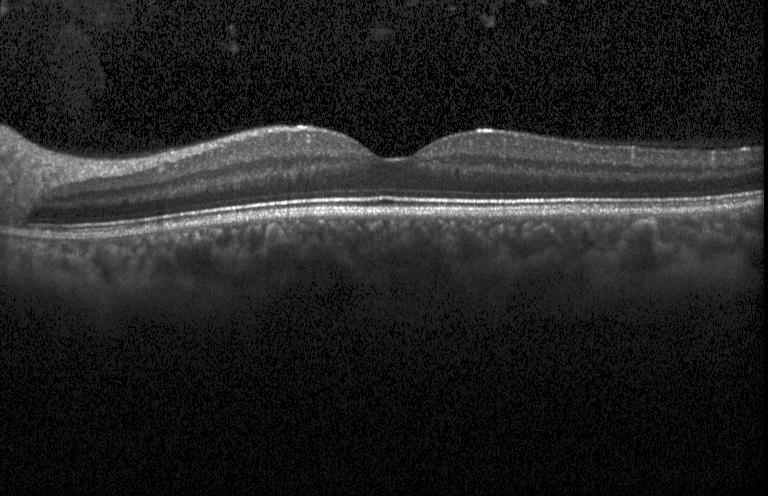

Optical coherence tomography B-scan
Dx: no choroidal neovascularization, no diabetic macular edema, and no drusen.